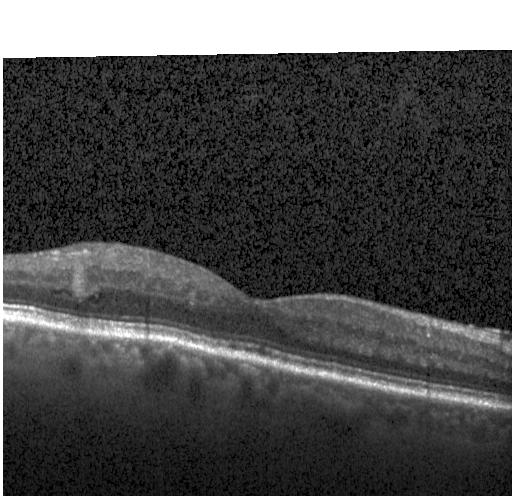 Optical coherence tomography scan. Finding: diabetic macular edema.